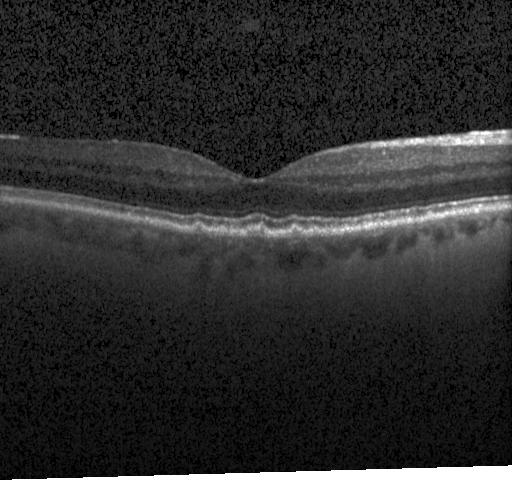

Retinal OCT cross-section, macular scan.
Finding: sub-RPE drusenoid deposits.